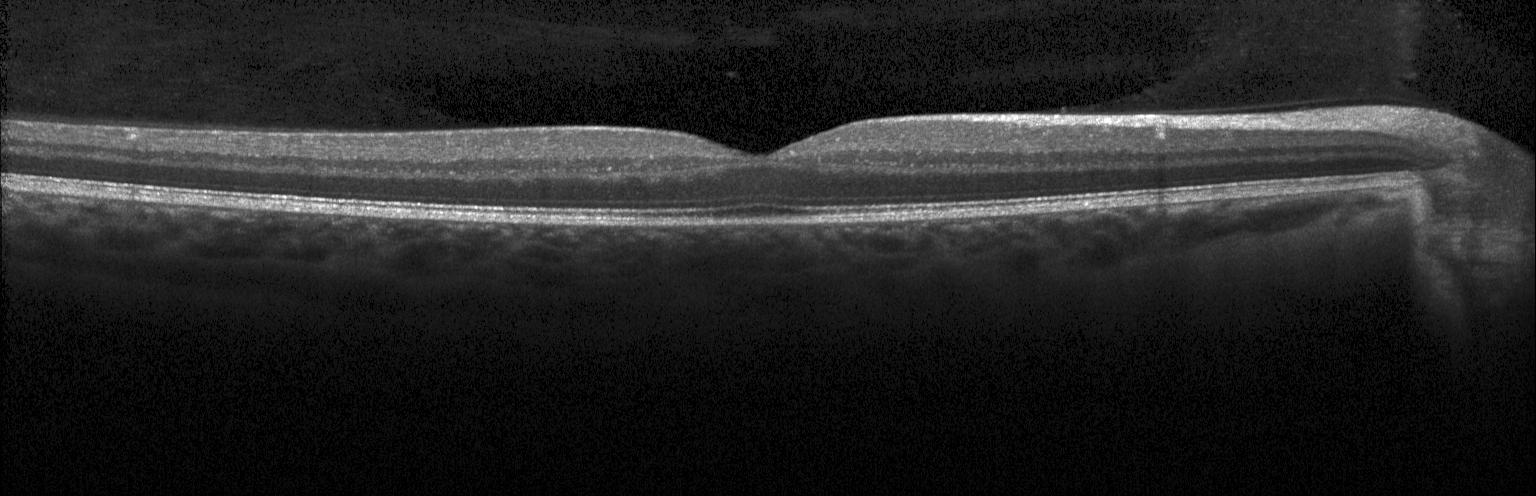
OCT B-scan · SD-OCT · acquired on a Heidelberg Spectralis · centered on the fovea.
Finding: no evidence of choroidal neovascularization, diabetic macular edema, or drusen.